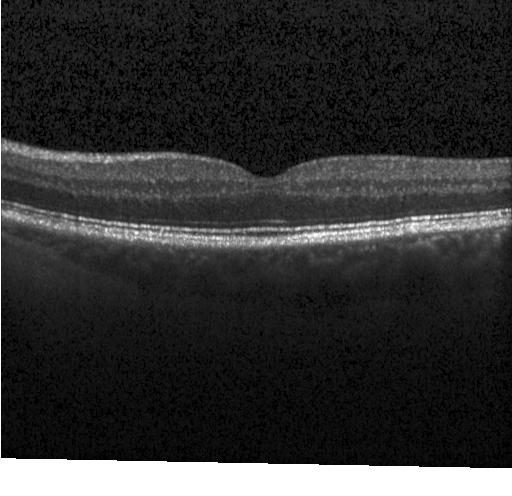
Neither choroidal neovascularization, diabetic macular edema, nor drusen.